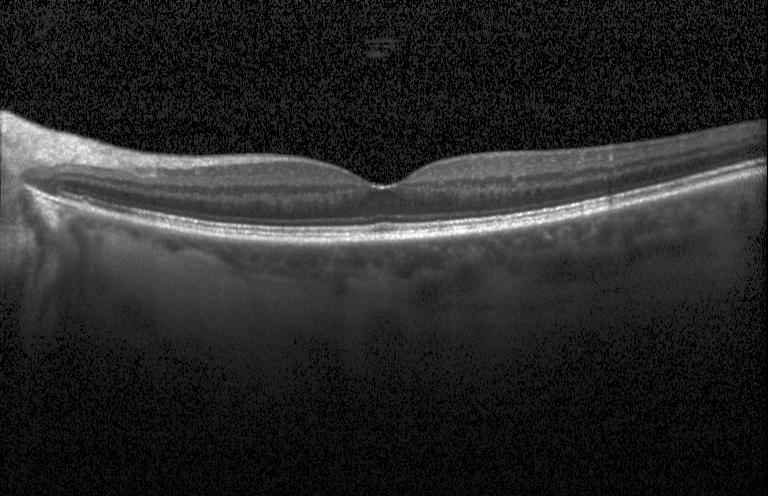 Instrument: Heidelberg Spectralis, spectral-domain OCT, retinal OCT cross-section.
Macular OCT: neither choroidal neovascularization, diabetic macular edema, nor drusen.